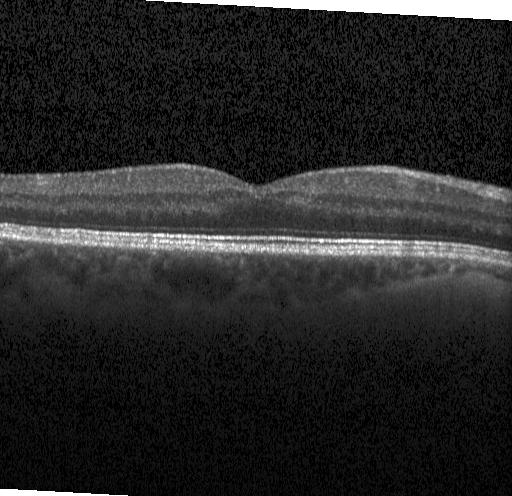
Spectral-domain OCT B-scan: neither choroidal neovascularization, diabetic macular edema, nor drusen.